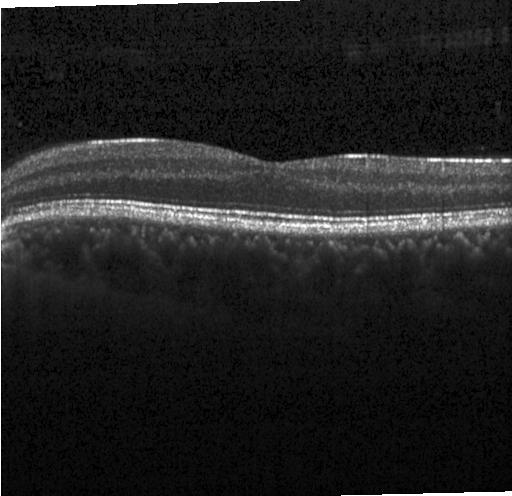 Centered on the fovea. OCT B-scan
Finding: no CNV, no DME, and no drusen.